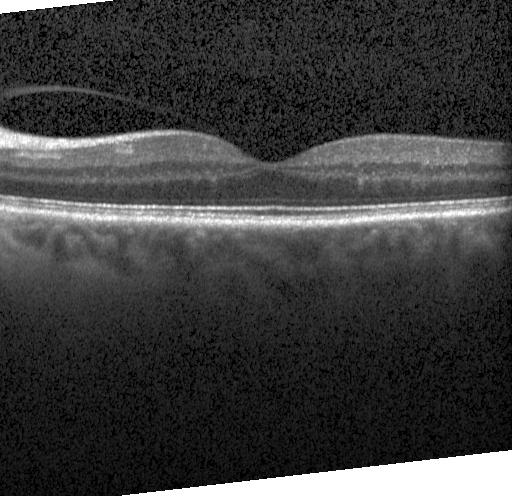

Diagnosis: neither CNV, DME, nor drusen.